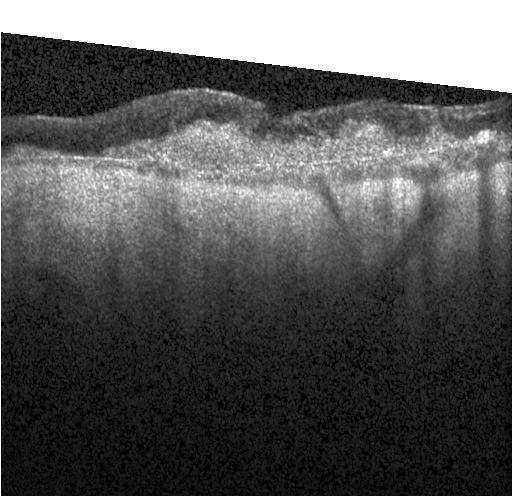
Retinal OCT cross-section
This B-scan demonstrates choroidal neovascularization (CNV).